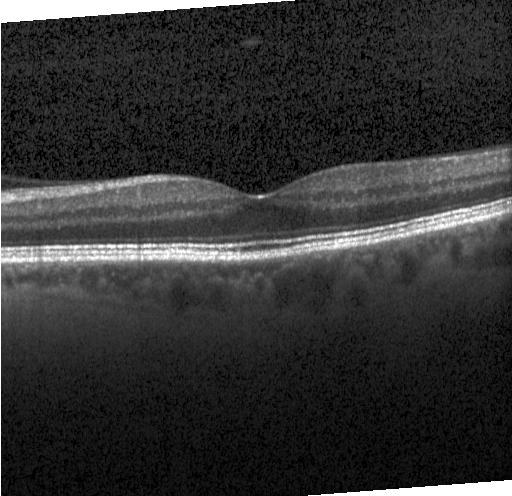

Heidelberg Spectralis. Fovea-centered. Retinal OCT B-scan. SD-OCT — Diagnosis: no choroidal neovascularization, diabetic macular edema, or drusen.